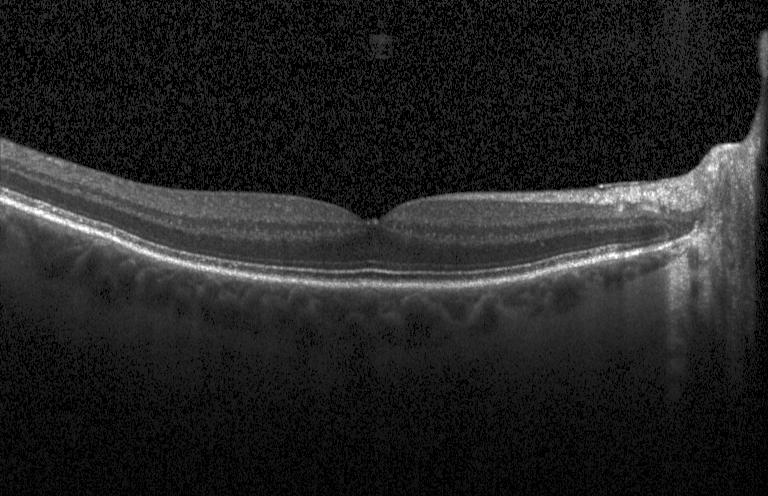

Retinal OCT cross-section.
Finding: neither choroidal neovascularization, diabetic macular edema, nor drusen.